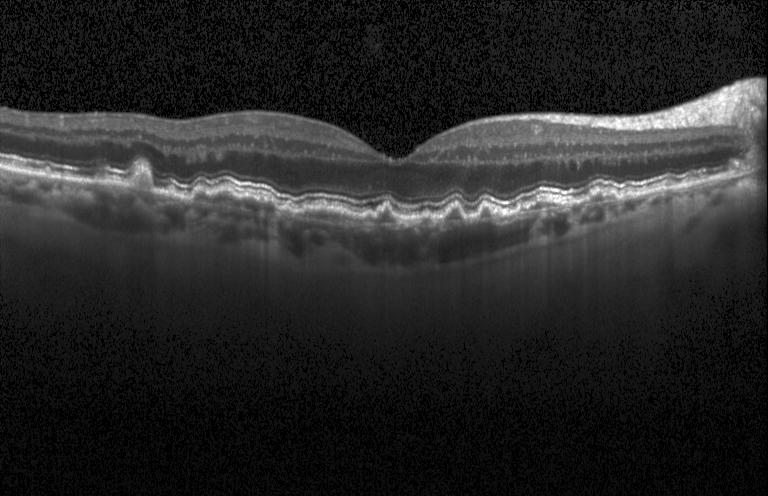 Retinal OCT cross-section showing sub-RPE drusenoid deposits.